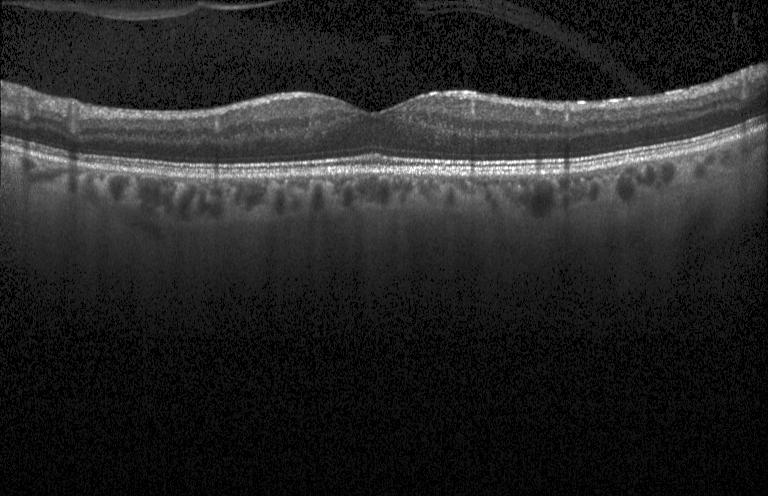
OCT scan showing neither choroidal neovascularization, diabetic macular edema, nor drusen.